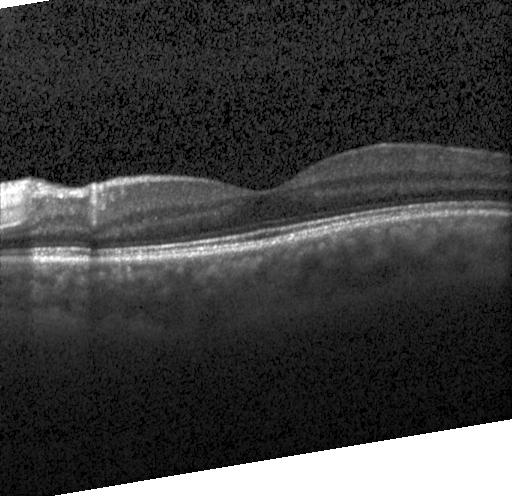 Spectral-domain OCT; OCT line scan; Heidelberg Spectralis. Diagnosis: no choroidal neovascularization, diabetic macular edema, or drusen.